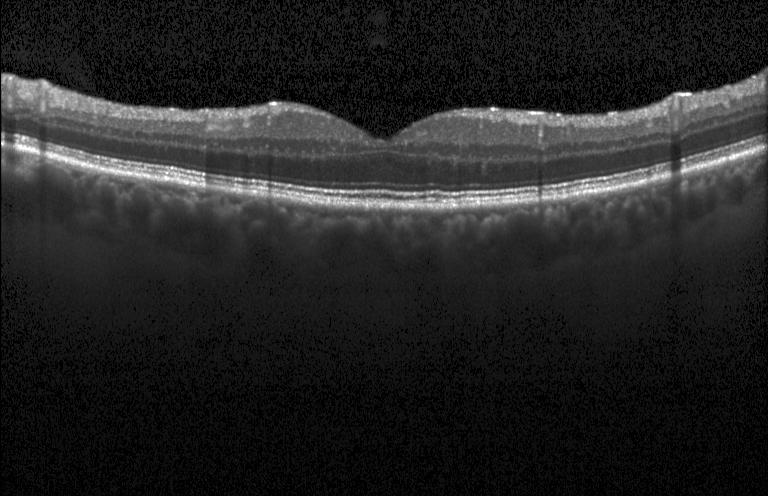
OCT B-scan, spectral-domain optical coherence tomography — Macular OCT: no choroidal neovascularization, no diabetic macular edema, and no drusen.